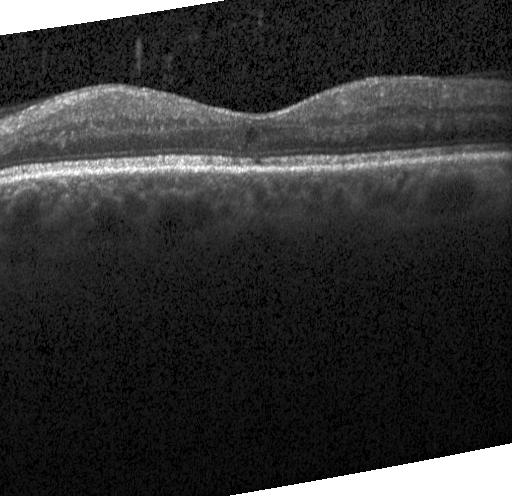
Impression: neither choroidal neovascularization, diabetic macular edema, nor drusen.